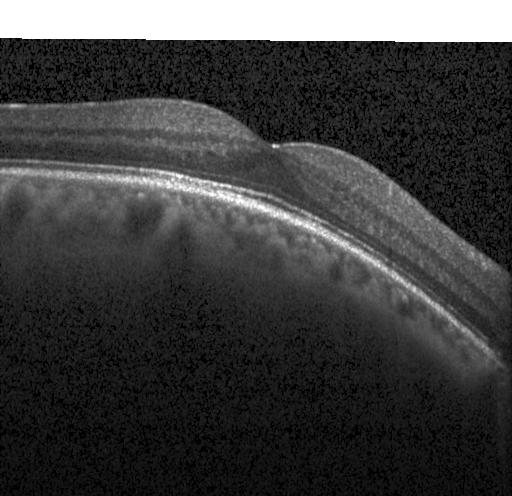
Centered on the fovea. Retinal OCT cross-section — No choroidal neovascularization, no diabetic macular edema, and no drusen.